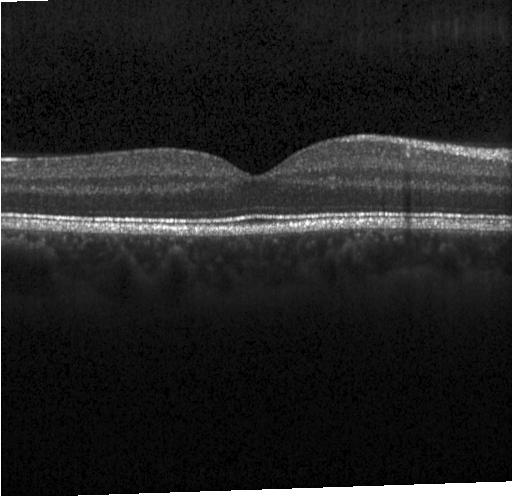 Through the macula · OCT B-scan · instrument: Heidelberg Spectralis · spectral-domain optical coherence tomography
Dx: no evidence of CNV, DME, or drusen.